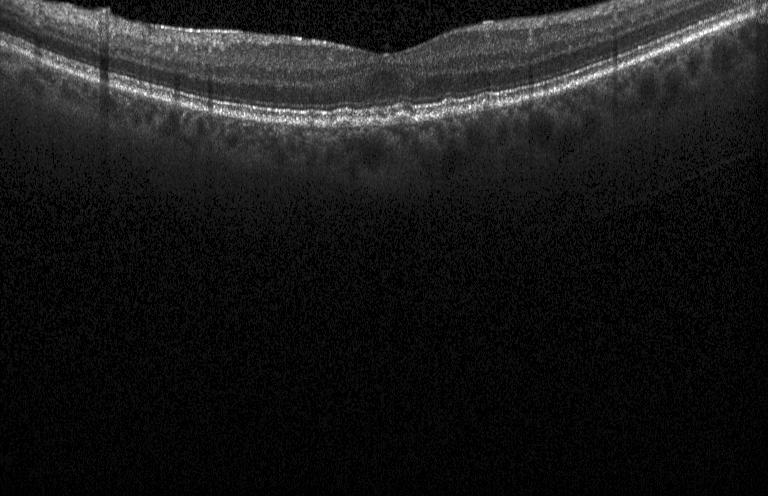
Through the macula; SD-OCT; OCT line scan; instrument: Heidelberg Spectralis
Impression: drusen.